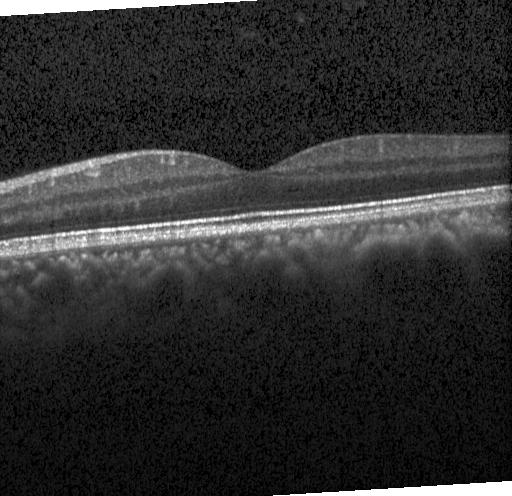

Optical coherence tomography scan
Dx: no CNV, DME, or drusen.